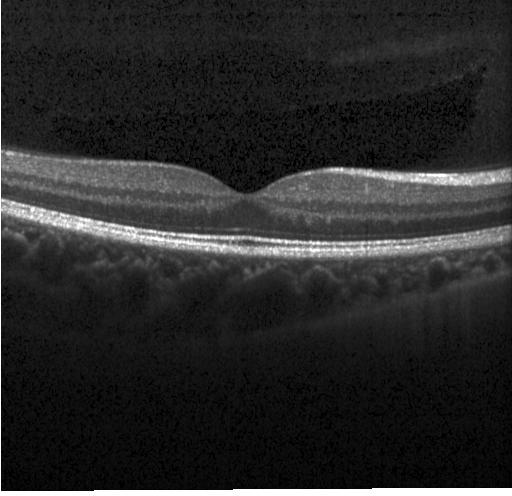
Centered on the fovea. OCT line scan. Heidelberg Spectralis OCT system.
Neither CNV, DME, nor drusen.